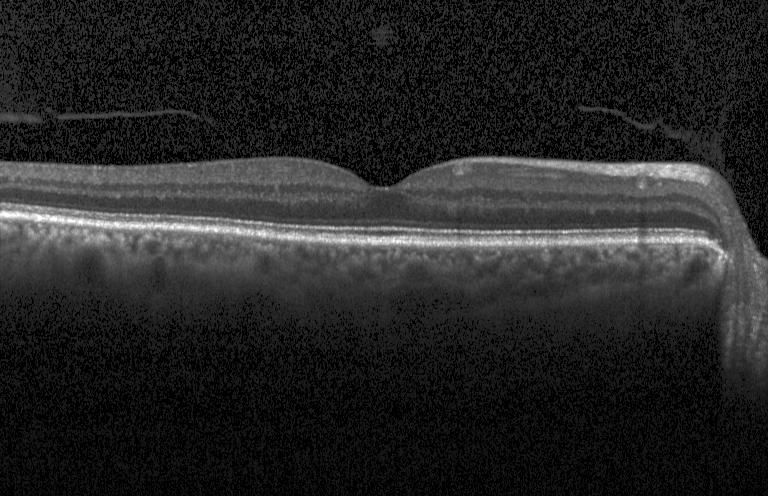
Impression: neither choroidal neovascularization, diabetic macular edema, nor drusen.